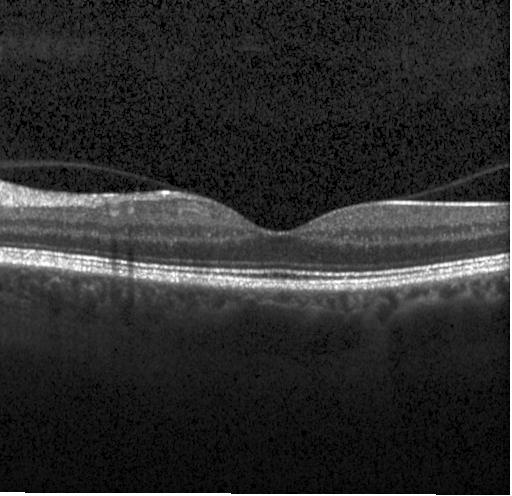

Spectral-domain OCT · OCT B-scan
Diagnosis: no evidence of CNV, DME, or drusen.